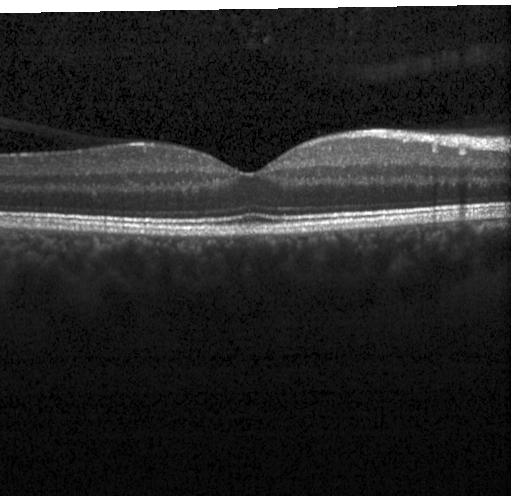

Acquired on a Heidelberg Spectralis; spectral-domain optical coherence tomography; fovea-centered; optical coherence tomography scan
Diagnosis: neither choroidal neovascularization, diabetic macular edema, nor drusen.